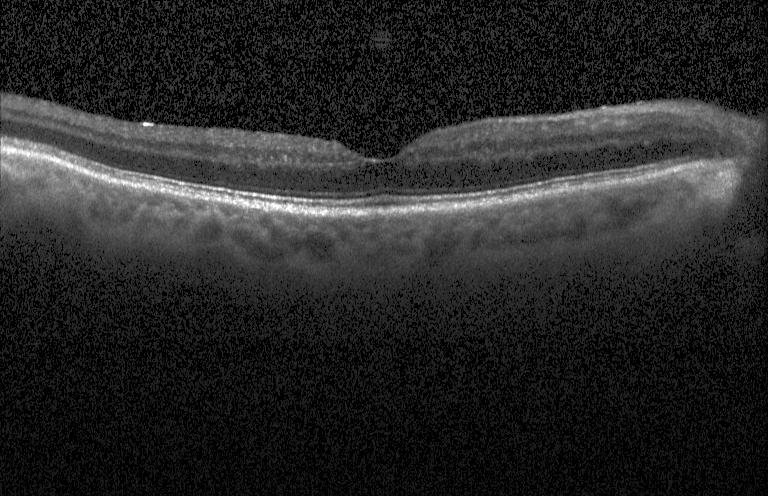 OCT B-scan showing no choroidal neovascularization, no diabetic macular edema, and no drusen.